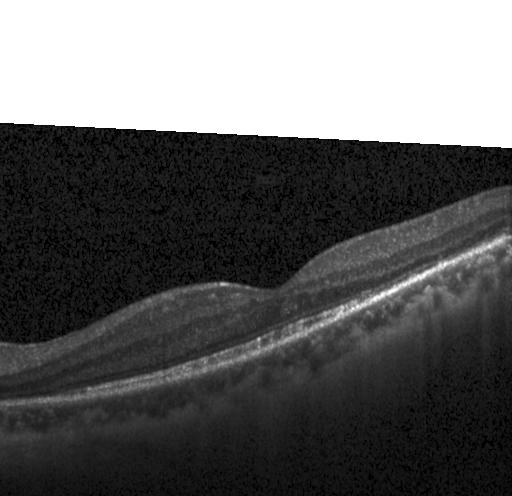 Centered on the fovea. Acquired on a Heidelberg Spectralis. Spectral-domain optical coherence tomography. OCT line scan. Diagnosis: no evidence of choroidal neovascularization, diabetic macular edema, or drusen.